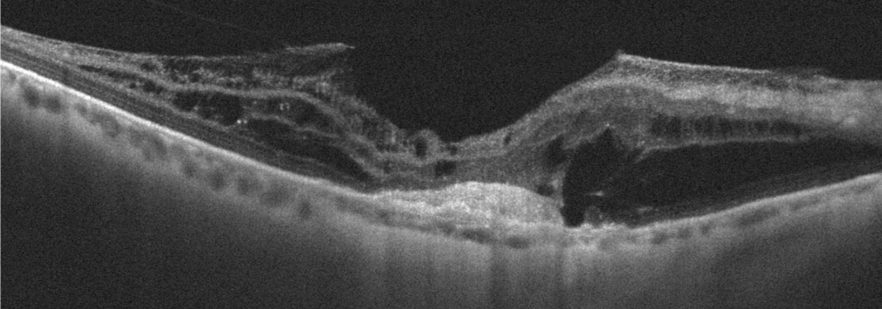

Finding: AMD.